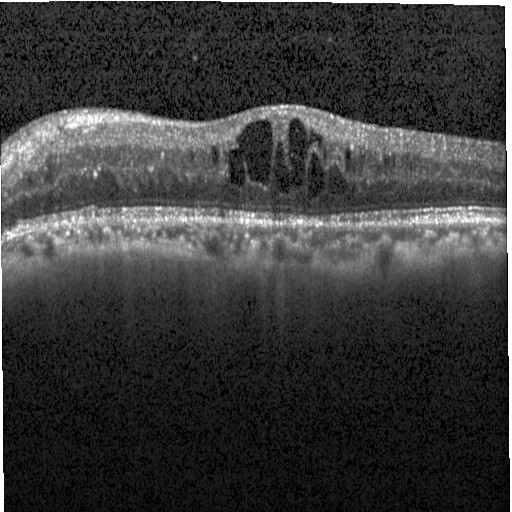
Spectral-domain optical coherence tomography · fovea-centered · optical coherence tomography B-scan · Heidelberg Spectralis. Macular OCT: DME.